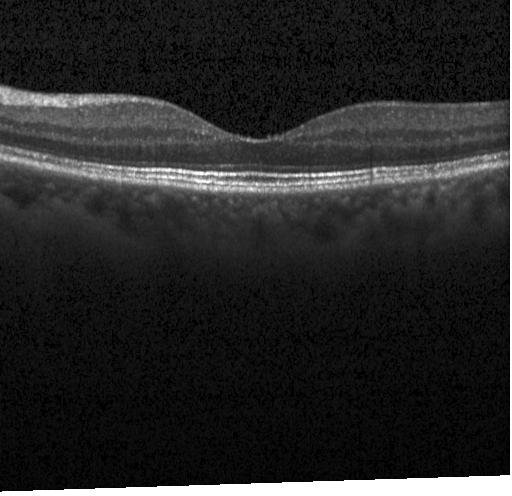 Centered on the fovea, OCT B-scan, spectral-domain OCT.
Diagnosis: no CNV, DME, or drusen.